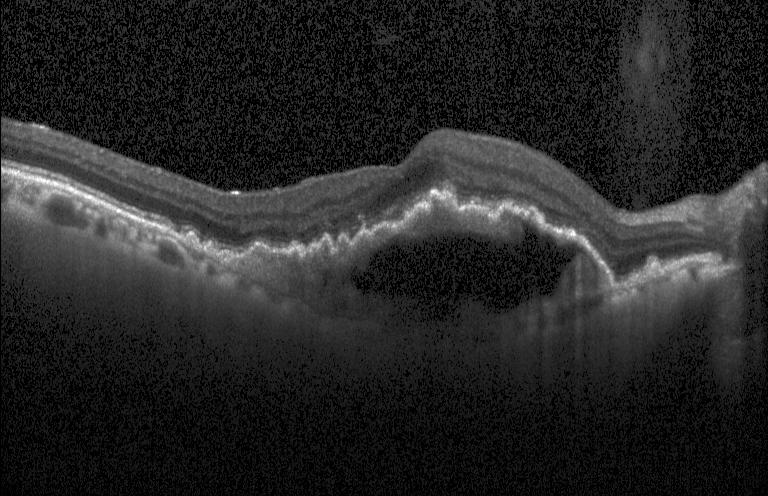
The scan shows a choroidal neovascular membrane.